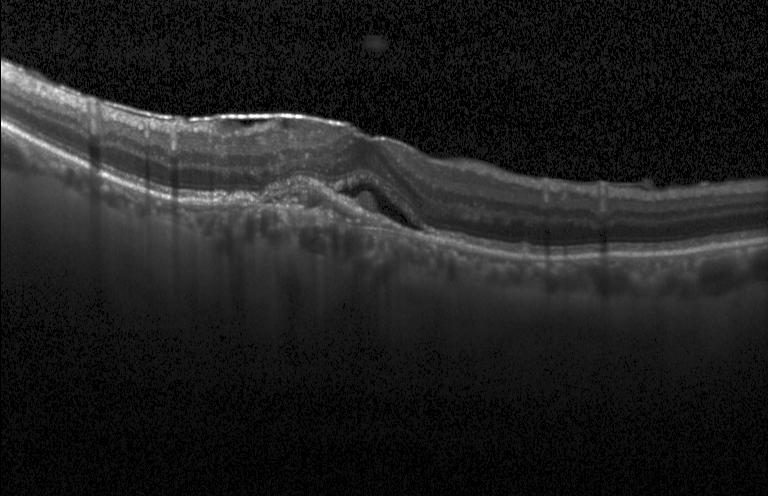

Macular OCT demonstrating a choroidal neovascular membrane.